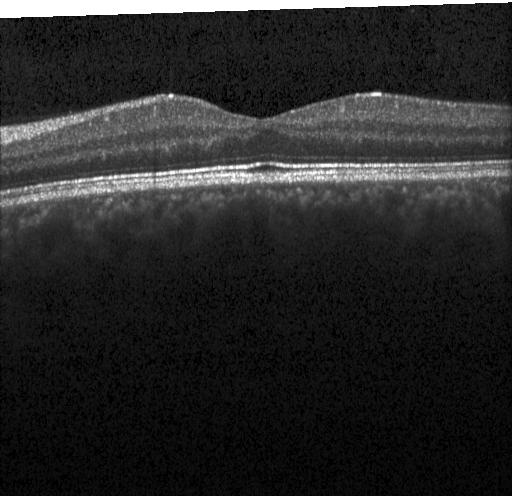
Acquired on a Heidelberg Spectralis; SD-OCT; retinal OCT cross-section; through the macula.
Finding: no choroidal neovascularization, diabetic macular edema, or drusen.